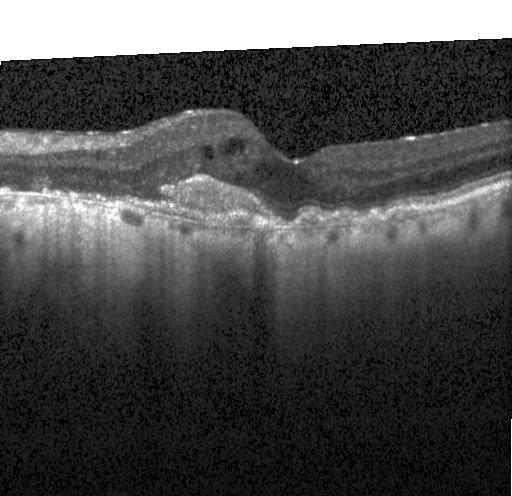 Macular OCT demonstrating a choroidal neovascular membrane.